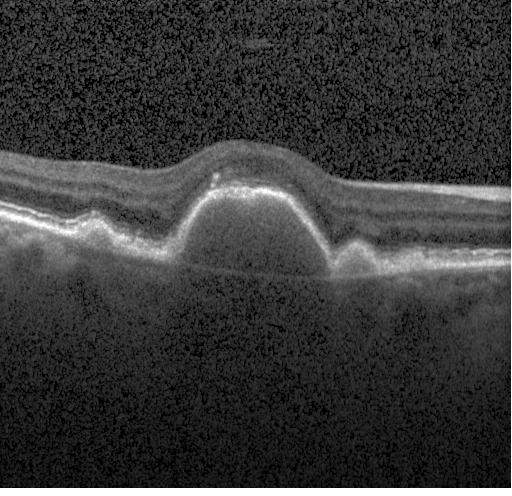

Retinal OCT cross-section; fovea-centered; spectral-domain optical coherence tomography; Heidelberg Spectralis OCT system.
Macular OCT: choroidal neovascularization (CNV).